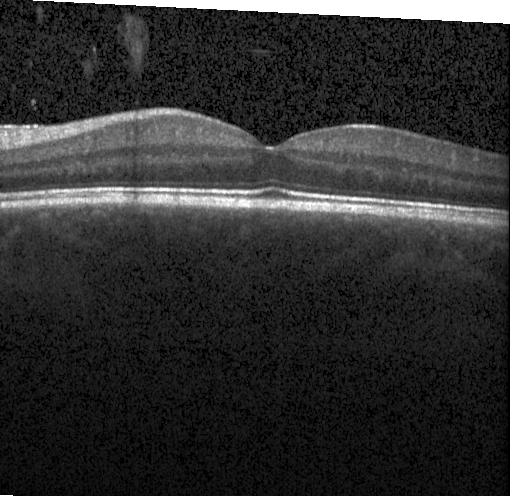 Optical coherence tomography scan
The scan shows no evidence of CNV, DME, or drusen.